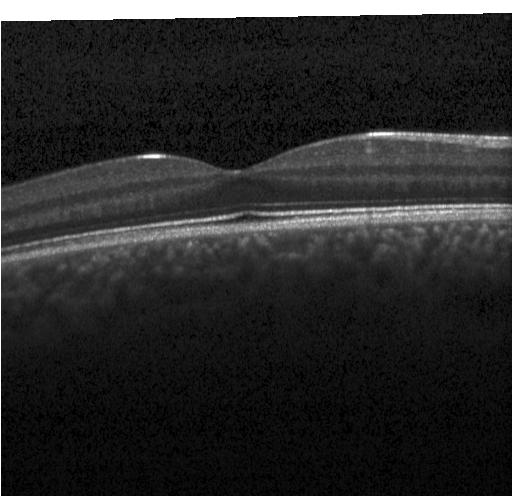

OCT line scan
Dx: no choroidal neovascularization, diabetic macular edema, or drusen.